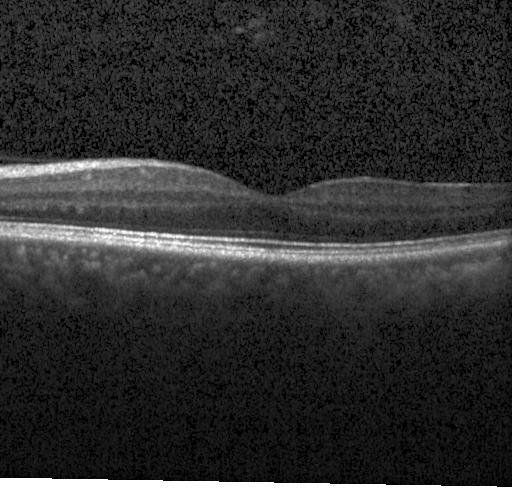
OCT scan showing no evidence of choroidal neovascularization, diabetic macular edema, or drusen.